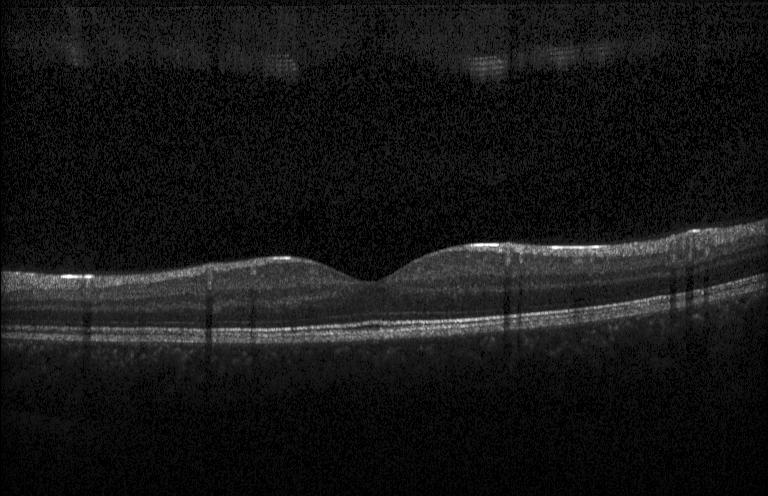 Instrument: Heidelberg Spectralis. Horizontal scan through the fovea. Spectral-domain optical coherence tomography. Optical coherence tomography scan.
Diagnosis: neither CNV, DME, nor drusen.